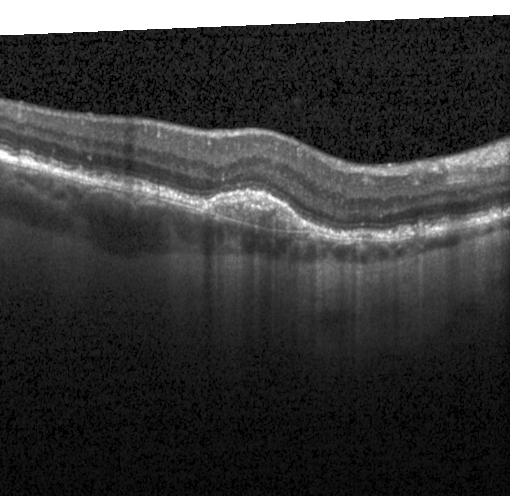
Optical coherence tomography B-scan
Finding: a choroidal neovascular membrane.